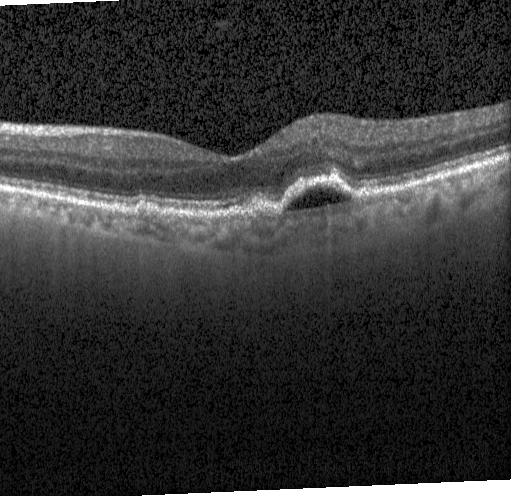 Retinal OCT cross-section; SD-OCT; horizontal scan through the fovea; acquired on a Heidelberg Spectralis — Assessment: choroidal neovascularization (CNV).